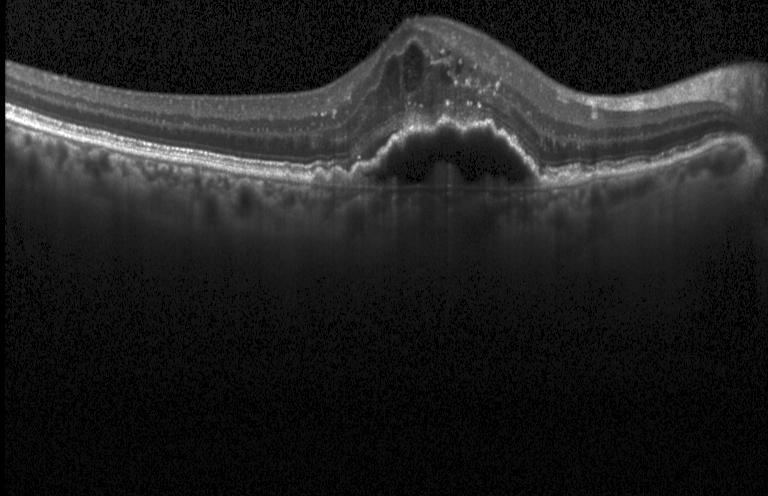 Macular scan; acquired on a Heidelberg Spectralis; OCT B-scan — OCT finding: CNV.